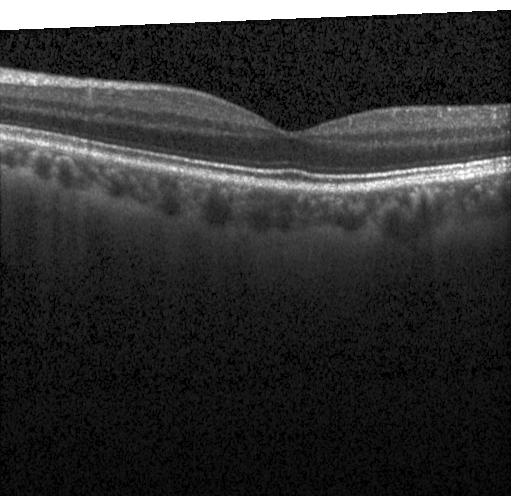
Macular OCT: no evidence of choroidal neovascularization, diabetic macular edema, or drusen.